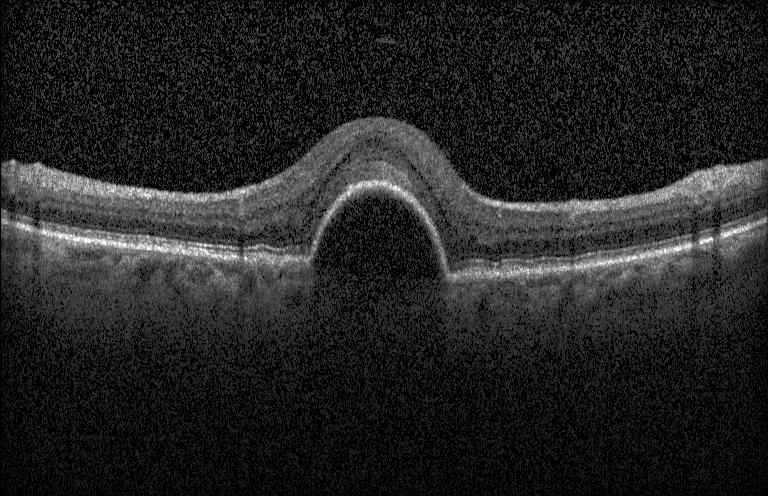

OCT line scan; spectral-domain OCT. Impression: CNV.